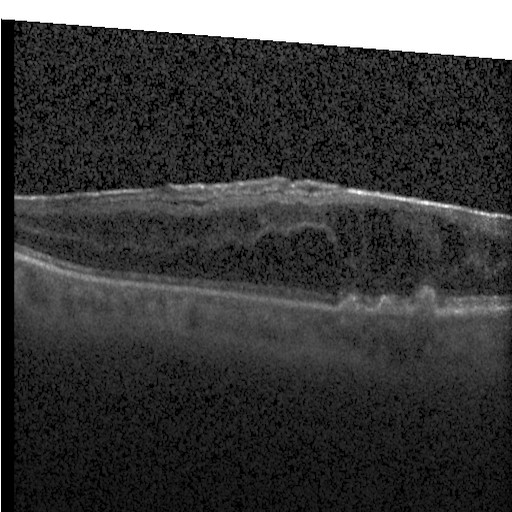

Heidelberg Spectralis; fovea-centered; SD-OCT; optical coherence tomography B-scan.
Diagnosis: diabetic macular edema.